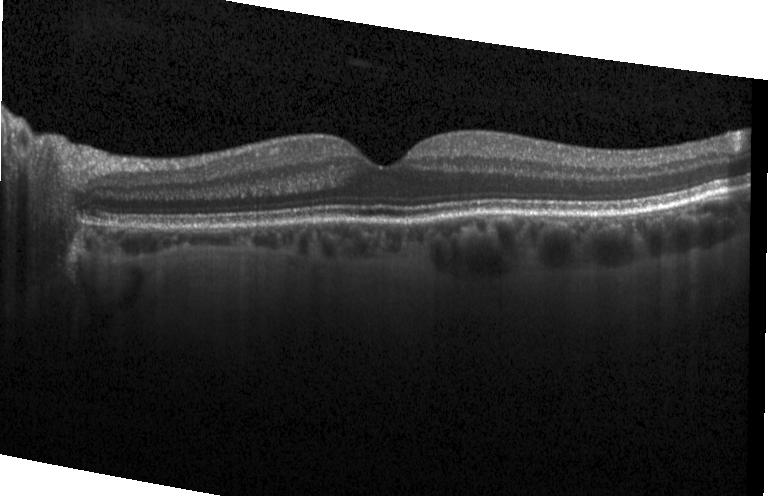
This B-scan demonstrates no evidence of choroidal neovascularization, diabetic macular edema, or drusen.